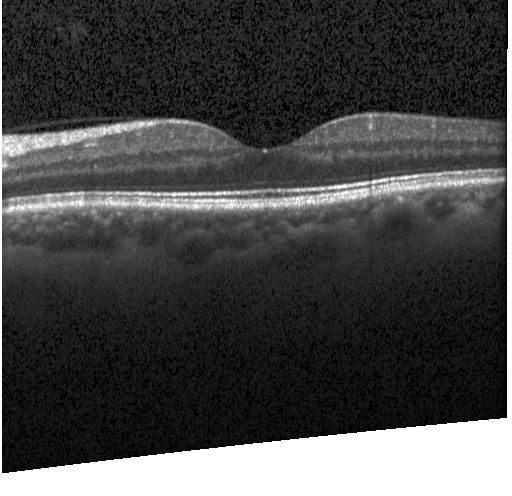
Horizontal scan through the fovea; retinal OCT cross-section; Heidelberg Spectralis OCT system; spectral-domain OCT
Dx: no choroidal neovascularization, diabetic macular edema, or drusen.